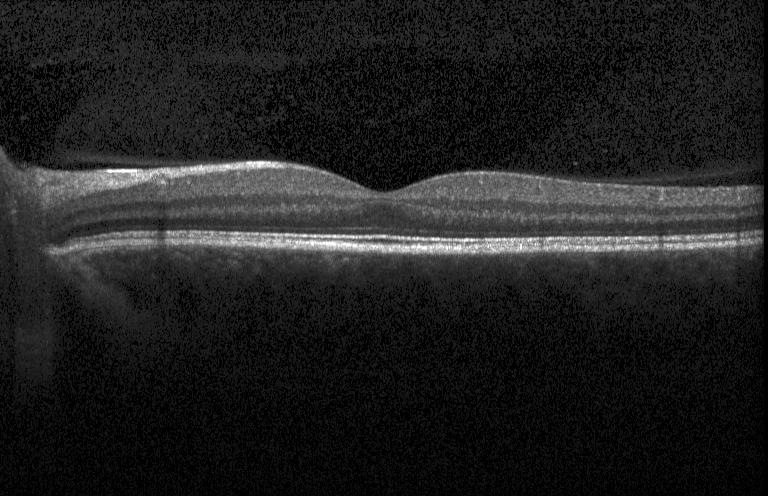

The scan shows no choroidal neovascularization, diabetic macular edema, or drusen.